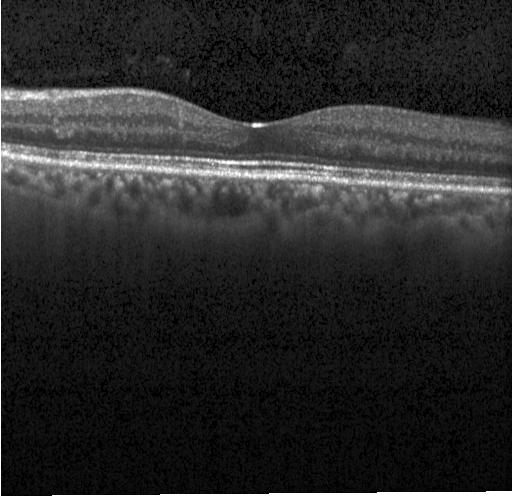
Heidelberg Spectralis; retinal OCT B-scan; macular scan; spectral-domain OCT — Finding: no CNV, DME, or drusen.